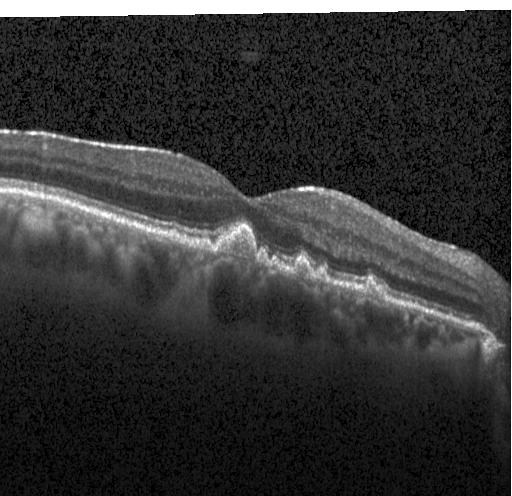
Heidelberg Spectralis; optical coherence tomography scan.
Diagnosis: drusen.